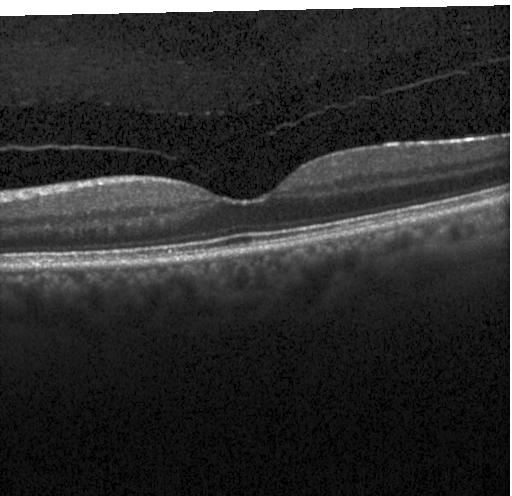 Retinal OCT cross-section. Heidelberg Spectralis.
Finding: neither CNV, DME, nor drusen.